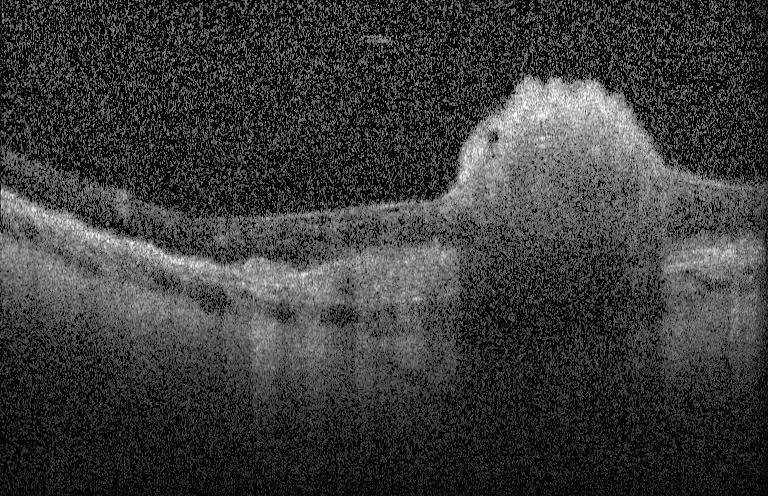 Horizontal scan through the fovea · optical coherence tomography B-scan · instrument: Heidelberg Spectralis — Dx: a choroidal neovascular membrane.